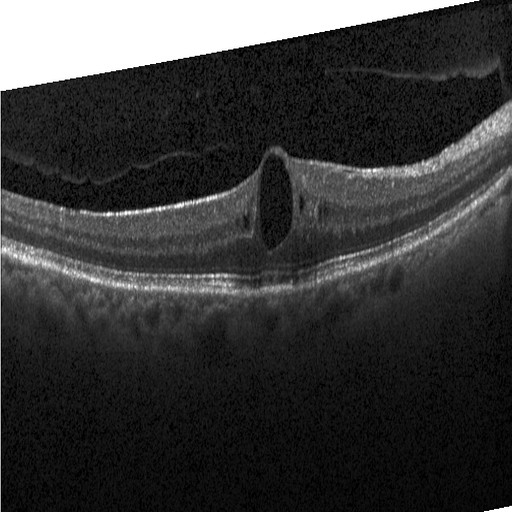 Macular OCT: diabetic macular edema (DME).